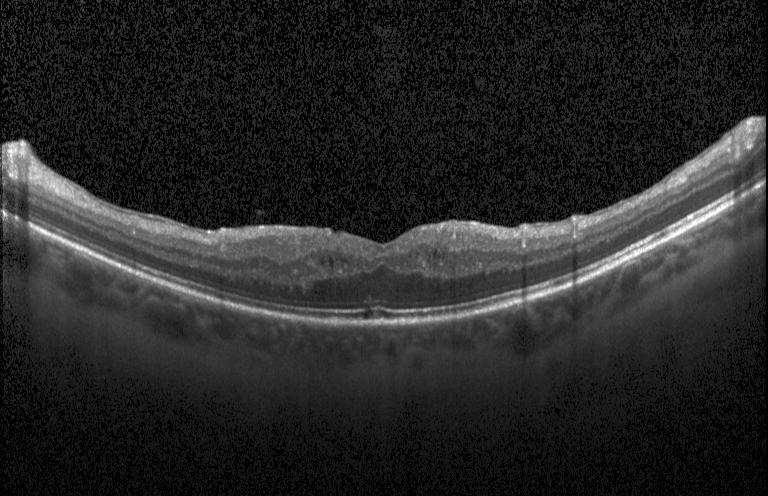

Acquired on a Heidelberg Spectralis, optical coherence tomography scan, SD-OCT, fovea-centered. OCT finding: diabetic macular edema.